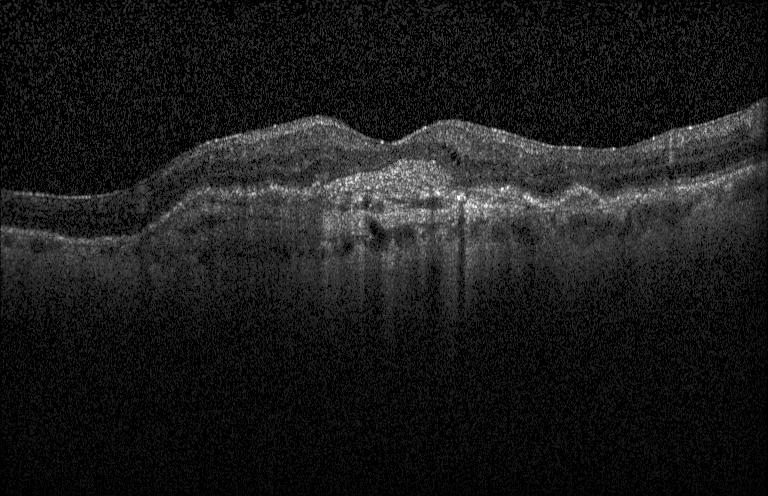

OCT line scan, Heidelberg Spectralis, spectral-domain OCT.
Finding: CNV.